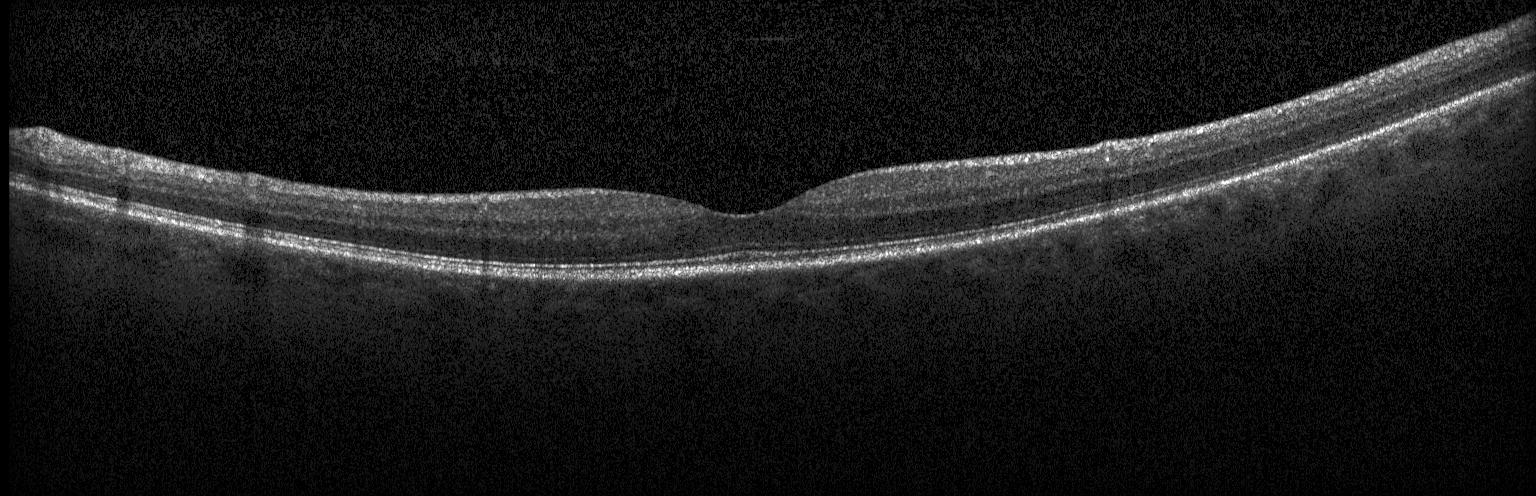 OCT B-scan showing no choroidal neovascularization, diabetic macular edema, or drusen.